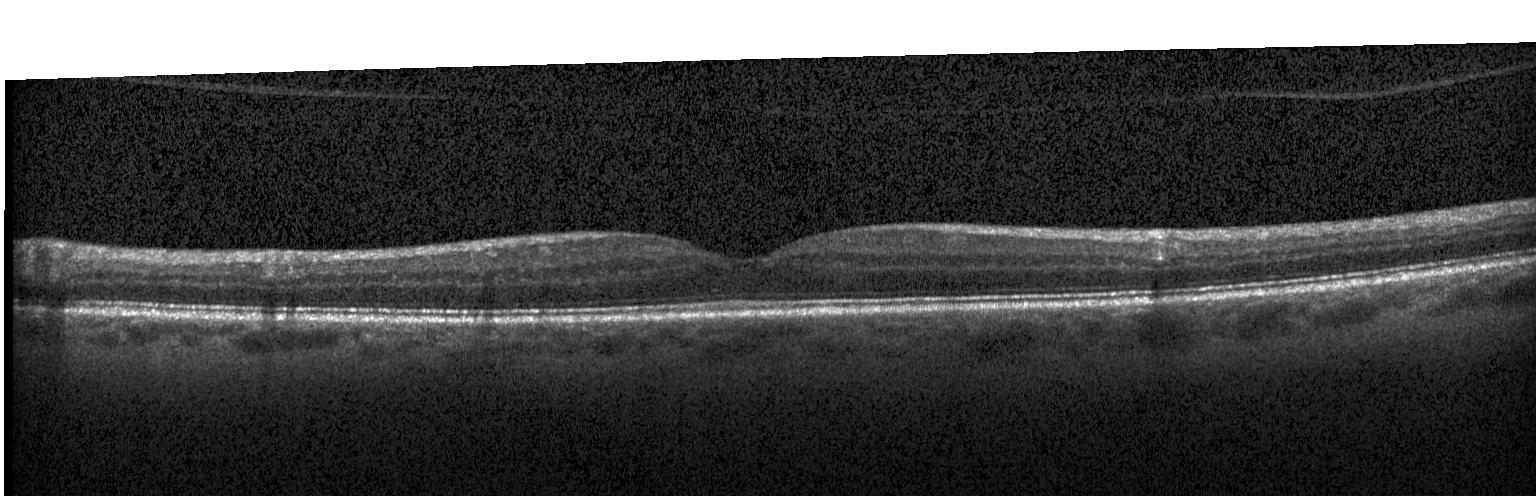
Spectral-domain optical coherence tomography · acquired on a Heidelberg Spectralis · macular scan · optical coherence tomography B-scan — Finding: no evidence of choroidal neovascularization, diabetic macular edema, or drusen.